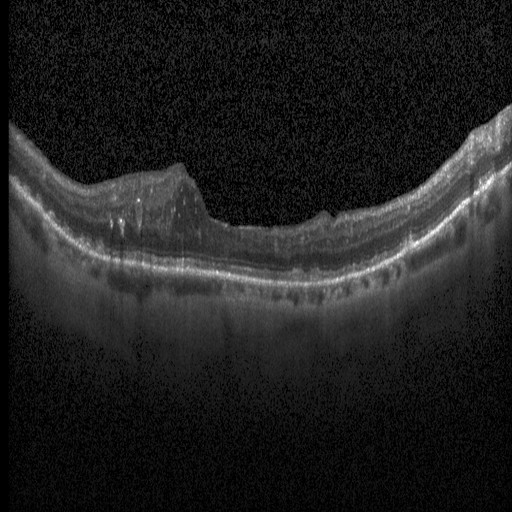

Retinal OCT B-scan. Diagnosis: diabetic macular edema.